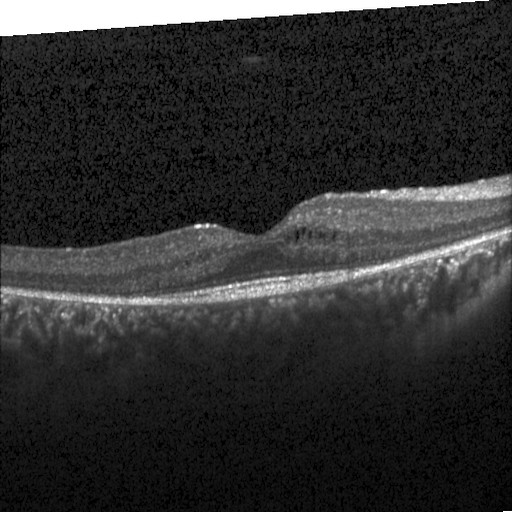
Acquired on a Heidelberg Spectralis; optical coherence tomography scan; macular scan. This B-scan demonstrates DME.